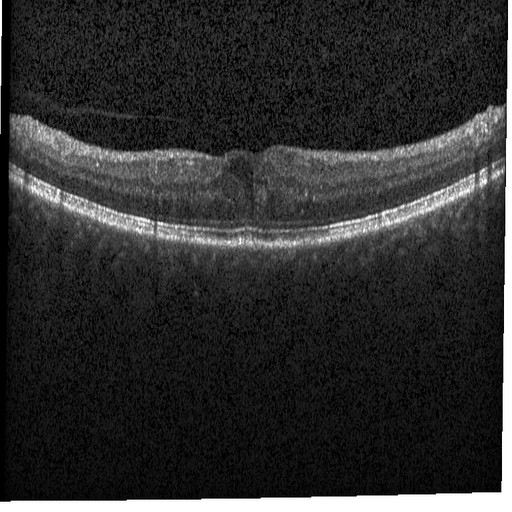
Impression: diabetic macular edema (DME).